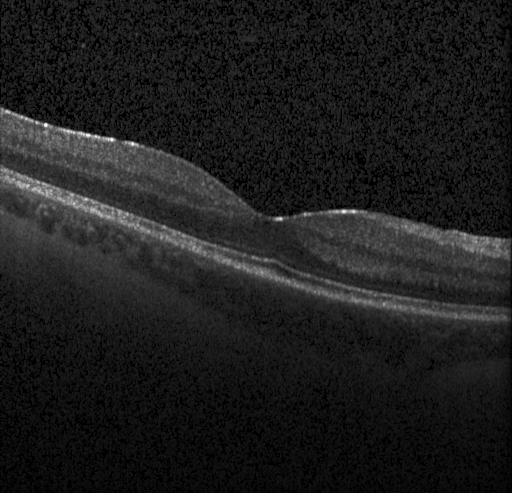 OCT line scan; SD-OCT; horizontal scan through the fovea; Heidelberg Spectralis — Finding: no CNV, no DME, and no drusen.